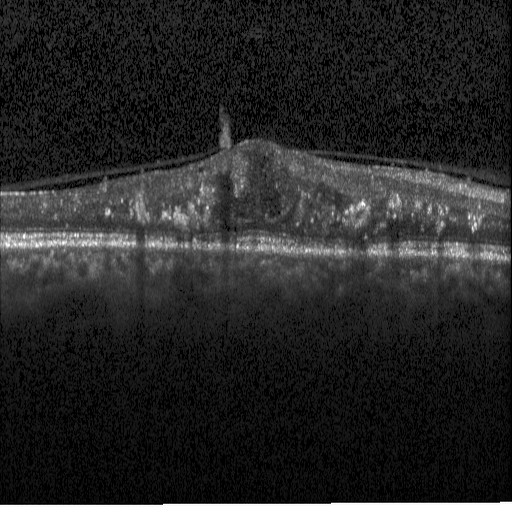
OCT scan showing diabetic macular edema (DME).